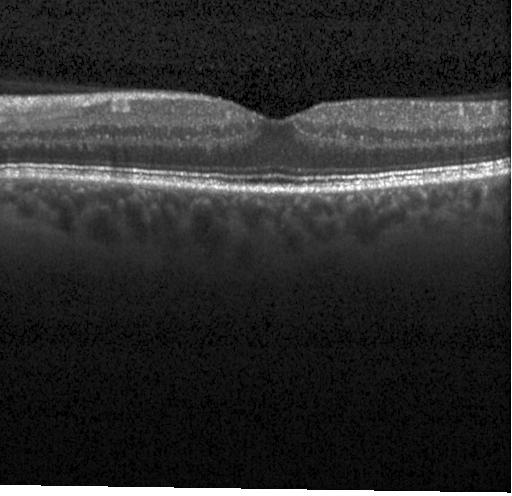

OCT finding: neither choroidal neovascularization, diabetic macular edema, nor drusen.